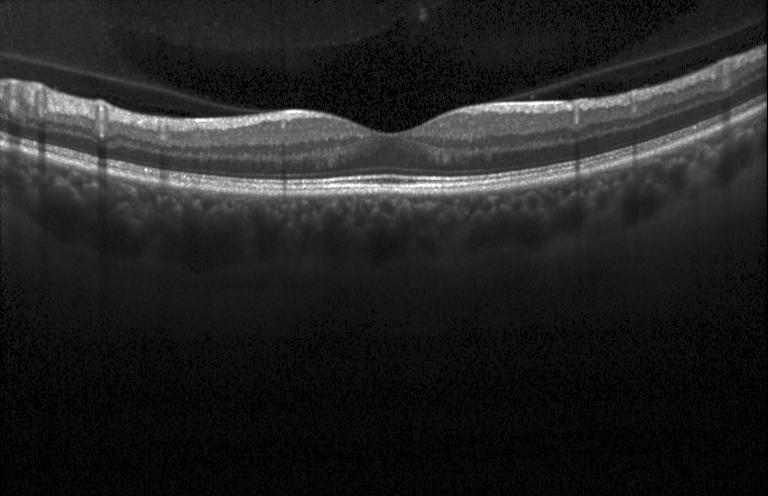 Finding: no choroidal neovascularization, diabetic macular edema, or drusen.